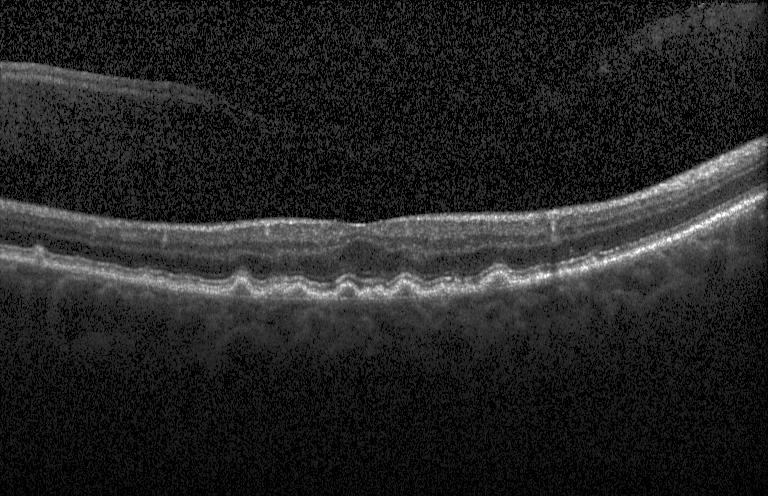

Finding: multiple drusen.